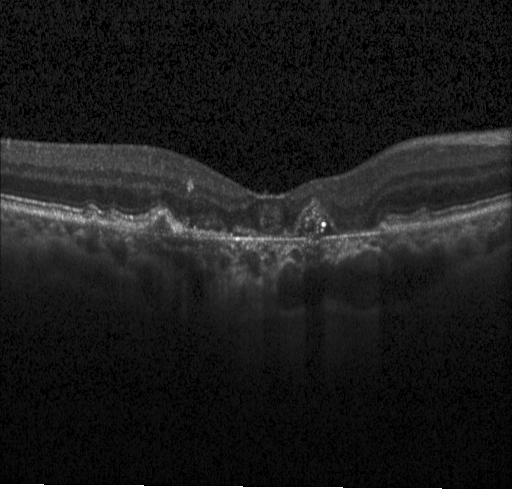
OCT scan showing CNV.